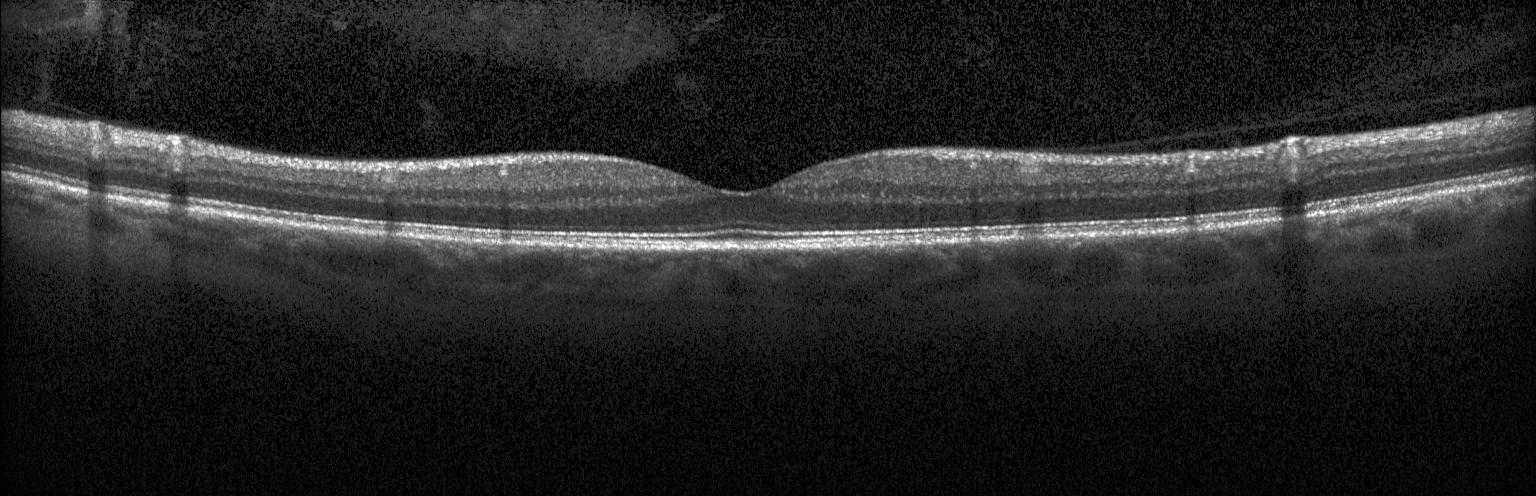

Fovea-centered; optical coherence tomography scan; acquired on a Heidelberg Spectralis; SD-OCT
Assessment: neither choroidal neovascularization, diabetic macular edema, nor drusen.